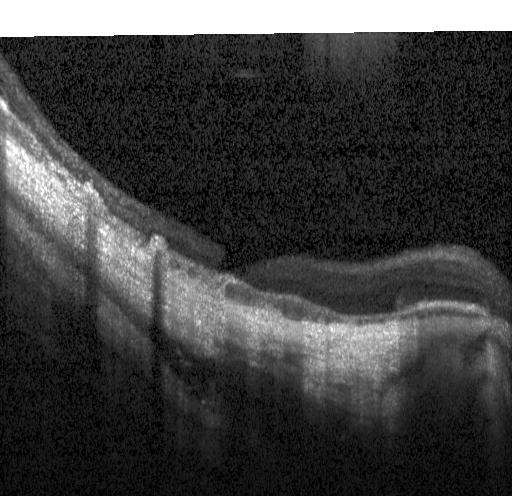 Spectral-domain OCT B-scan: a choroidal neovascular membrane.